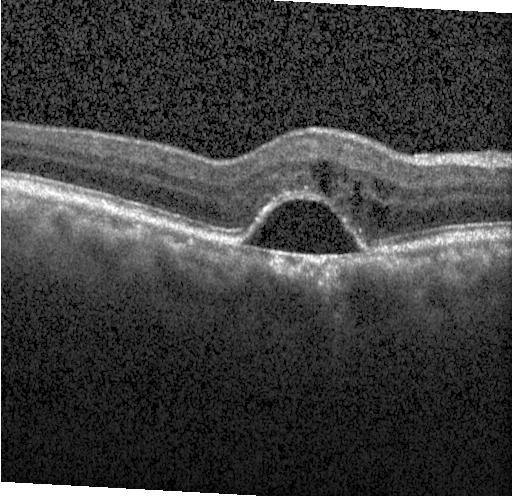

Retinal OCT cross-section showing choroidal neovascularization.